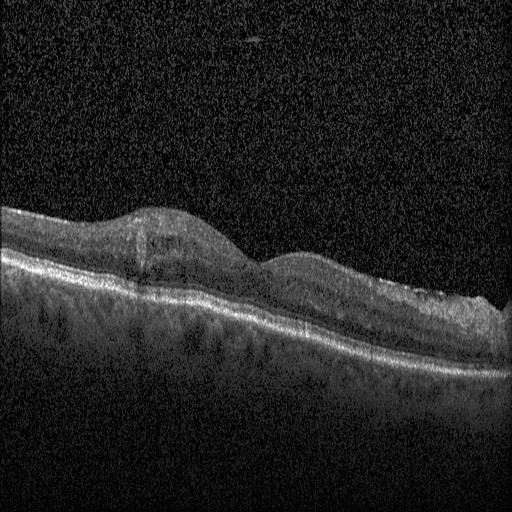
Dx: diabetic macular edema (DME).